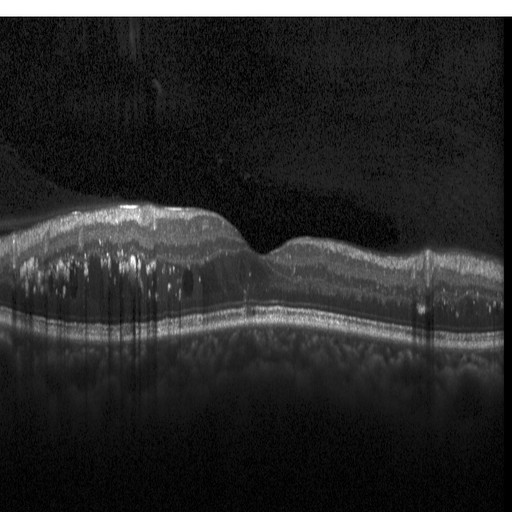

Diagnosis: diabetic macular edema (DME).